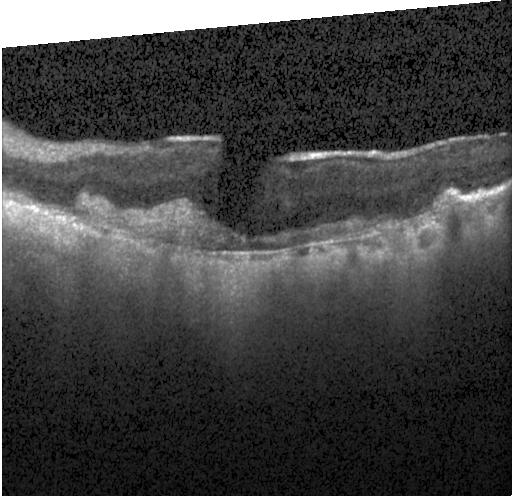

Spectral-domain optical coherence tomography; horizontal scan through the fovea; retinal OCT cross-section; acquired on a Heidelberg Spectralis.
This B-scan demonstrates a choroidal neovascular membrane.